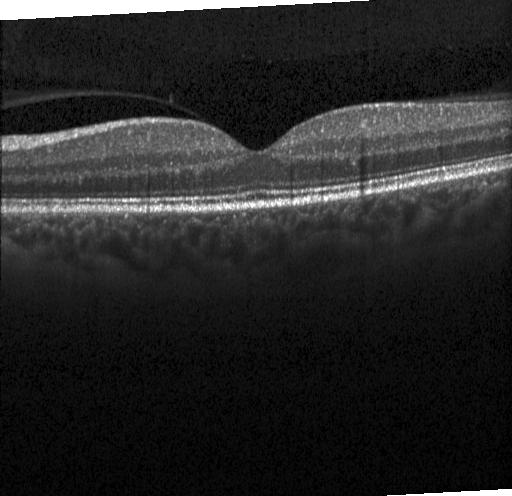
Centered on the fovea; OCT B-scan.
Diagnosis: neither choroidal neovascularization, diabetic macular edema, nor drusen.